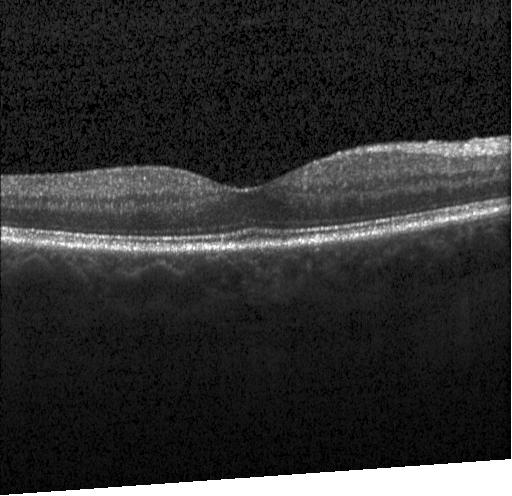 Heidelberg Spectralis · retinal OCT B-scan · macular scan. The scan shows no evidence of choroidal neovascularization, diabetic macular edema, or drusen.